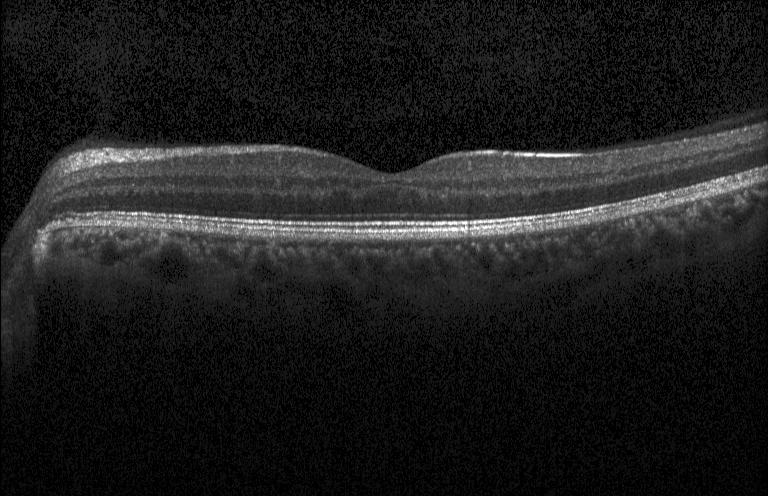
This B-scan demonstrates no evidence of CNV, DME, or drusen.